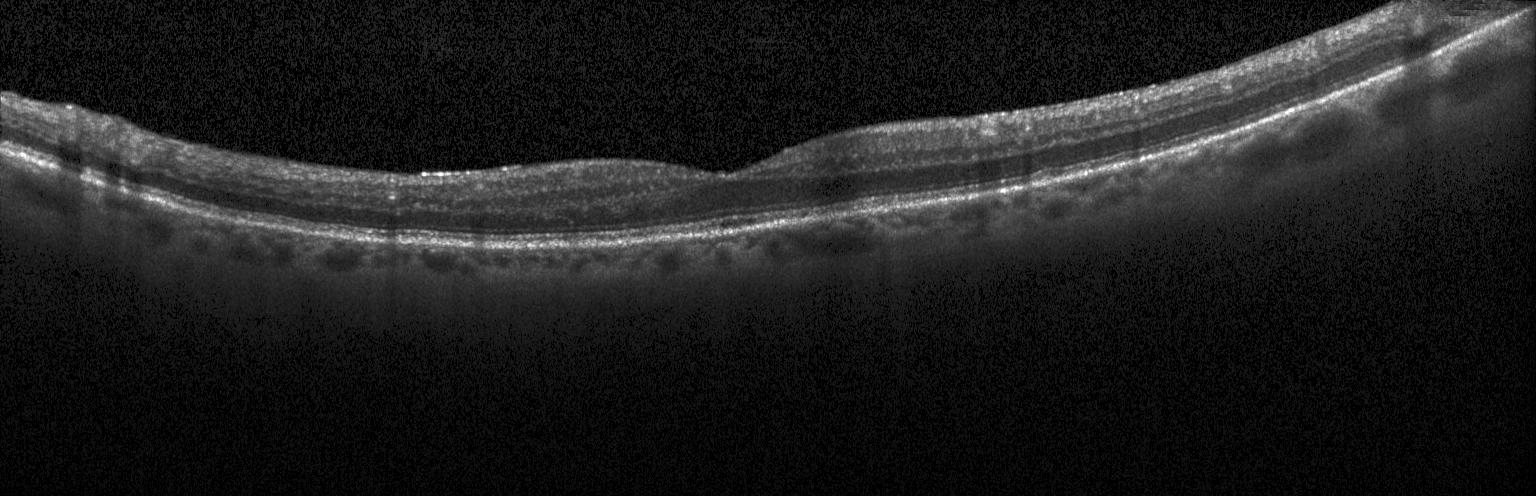
Centered on the fovea. Acquired on a Heidelberg Spectralis. OCT B-scan
OCT finding: no evidence of choroidal neovascularization, diabetic macular edema, or drusen.